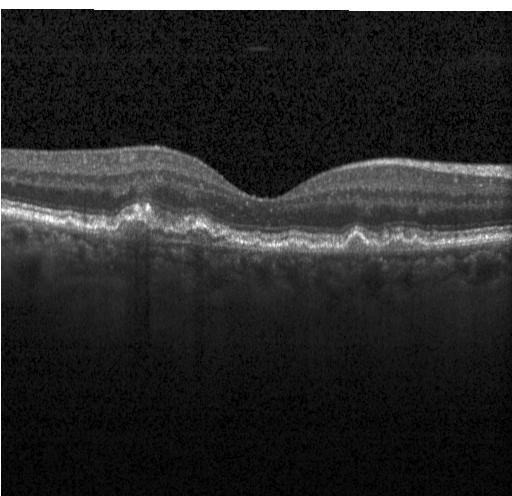 Retinal OCT B-scan · SD-OCT · instrument: Heidelberg Spectralis · horizontal scan through the fovea. Macular OCT: CNV.